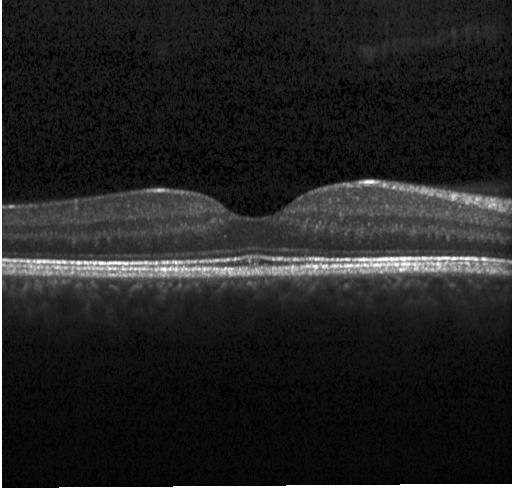 OCT finding: no choroidal neovascularization, no diabetic macular edema, and no drusen.